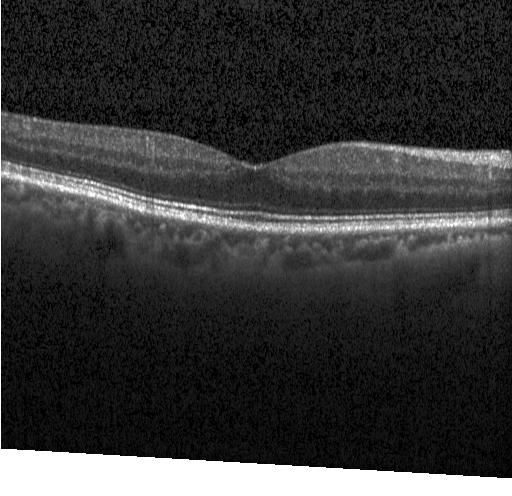
Heidelberg Spectralis · optical coherence tomography B-scan · spectral-domain OCT · horizontal scan through the fovea. This B-scan demonstrates no CNV, DME, or drusen.